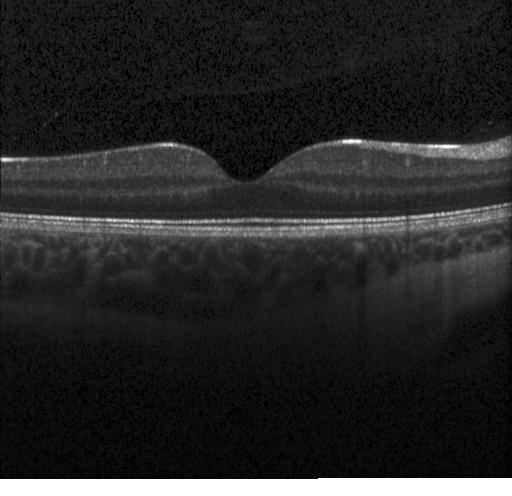
This B-scan demonstrates no choroidal neovascularization, no diabetic macular edema, and no drusen.